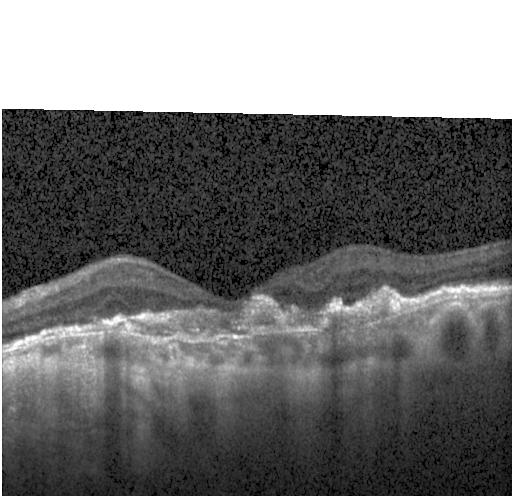
Impression: CNV.